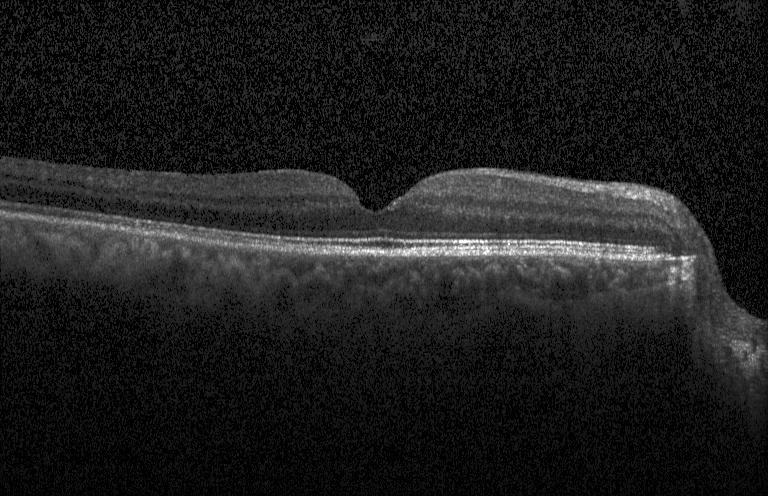
Impression: no CNV, DME, or drusen.